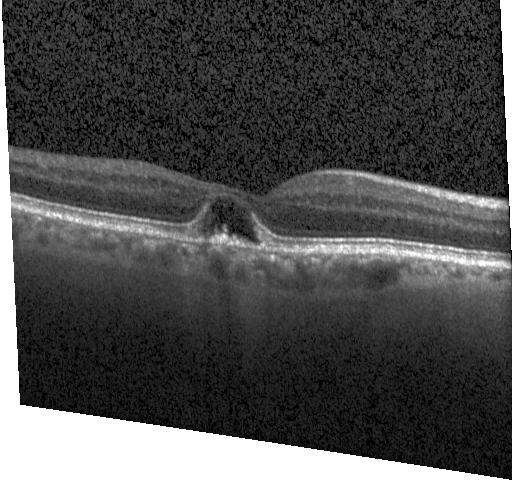 Retinal OCT B-scan, horizontal scan through the fovea. Macular OCT: choroidal neovascularization (CNV).